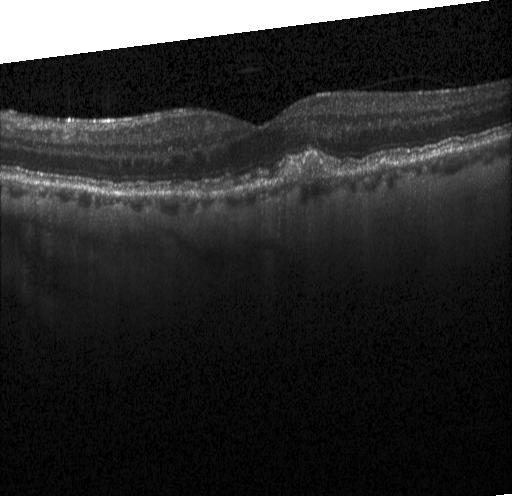

Macular OCT: multiple drusen.